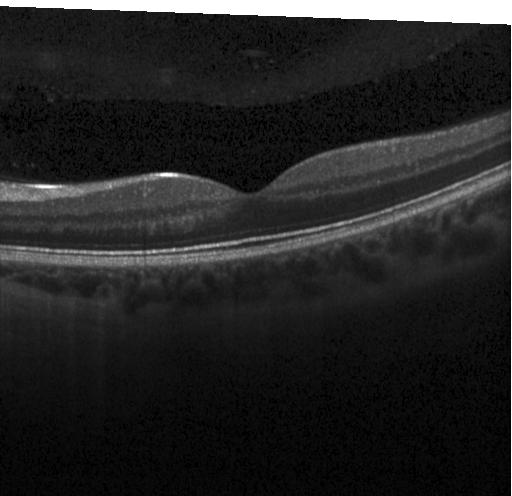 Instrument: Heidelberg Spectralis. Retinal OCT B-scan. This B-scan demonstrates no evidence of choroidal neovascularization, diabetic macular edema, or drusen.